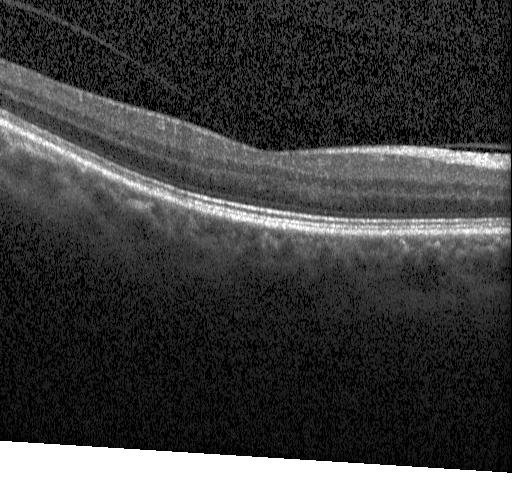 Acquired on a Heidelberg Spectralis, retinal OCT cross-section — Macular OCT: no choroidal neovascularization, diabetic macular edema, or drusen.